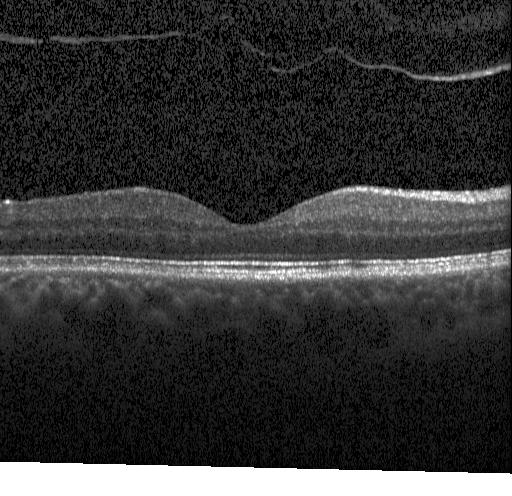

Retinal OCT cross-section — No evidence of choroidal neovascularization, diabetic macular edema, or drusen.